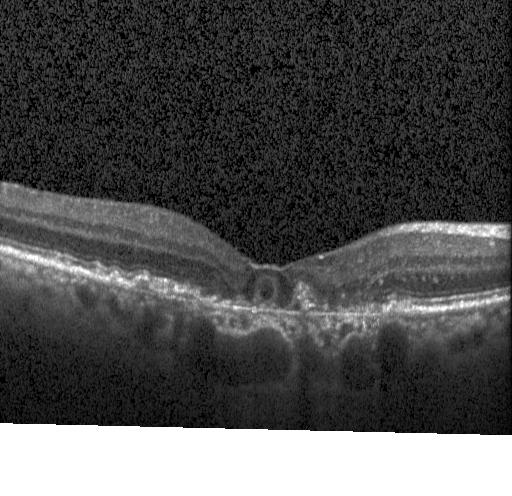
Assessment: choroidal neovascularization.